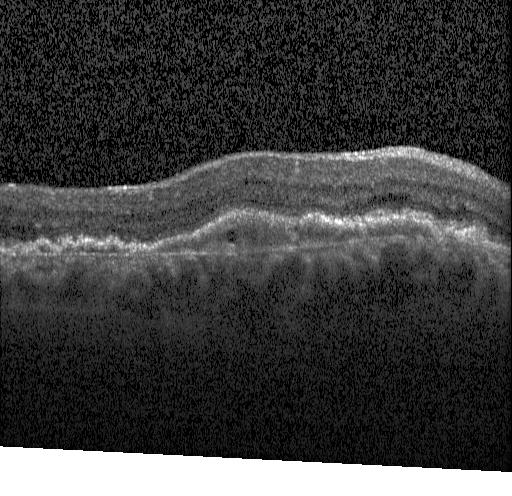
Macular OCT demonstrating a choroidal neovascular membrane.